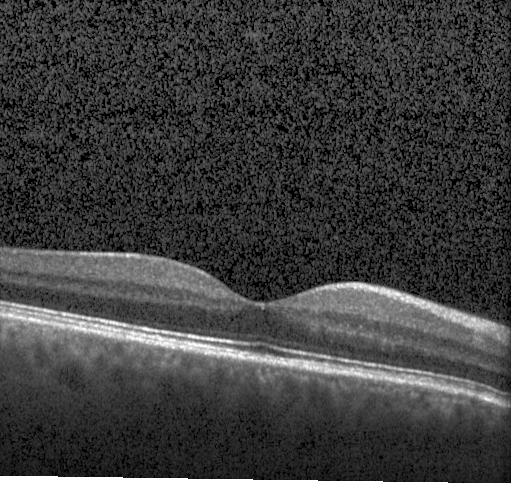 Retinal OCT B-scan; spectral-domain optical coherence tomography; acquired on a Heidelberg Spectralis; horizontal scan through the fovea
Diagnosis: neither CNV, DME, nor drusen.